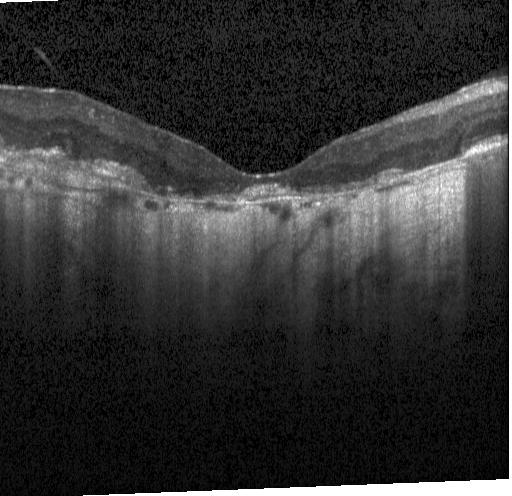
Macular OCT demonstrating choroidal neovascularization (CNV).